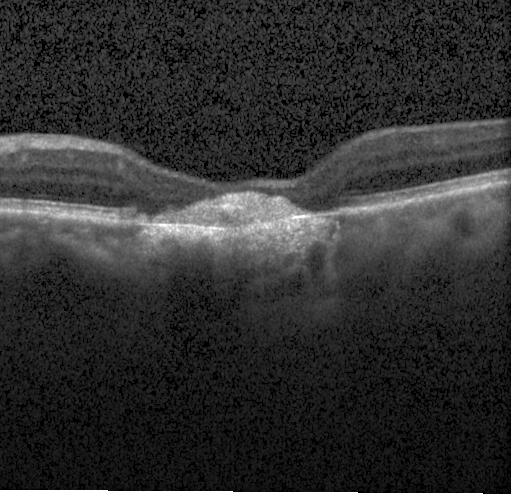 Instrument: Heidelberg Spectralis · centered on the fovea · OCT B-scan
The scan shows CNV.